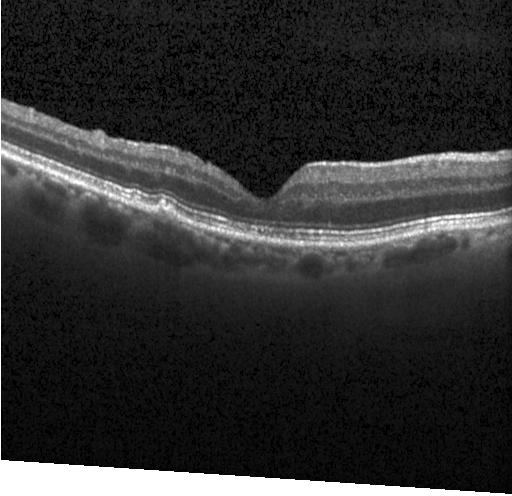

Retinal OCT cross-section · horizontal scan through the fovea — Impression: sub-RPE drusenoid deposits.